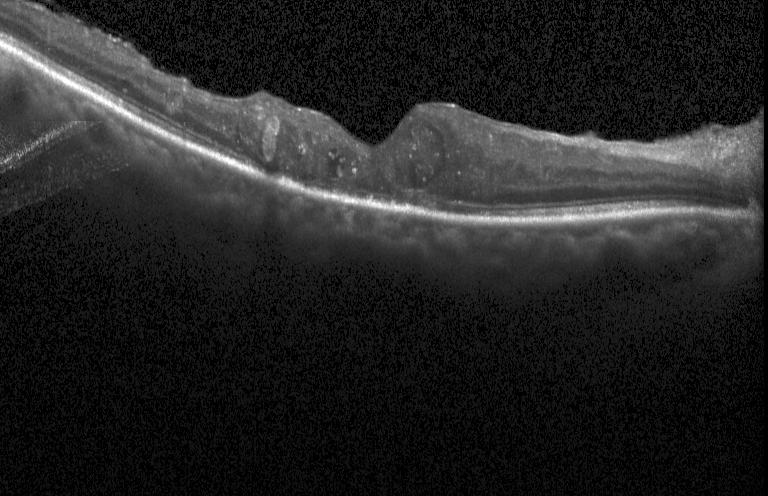 Retinal OCT cross-section showing diabetic macular edema.